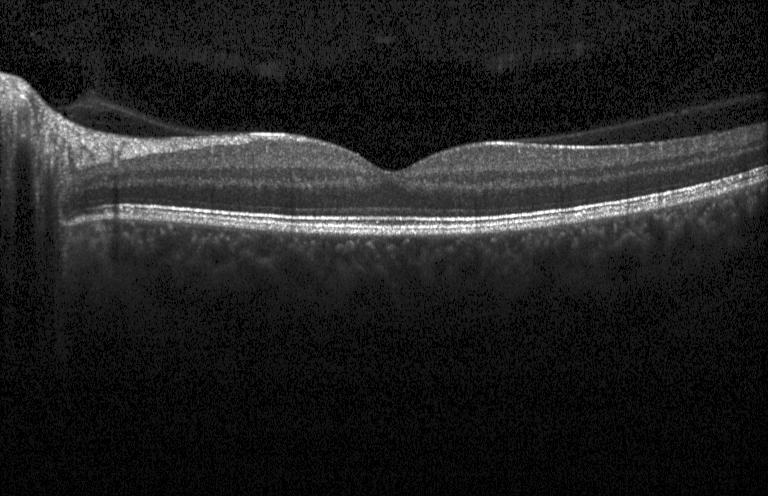
Heidelberg Spectralis; retinal OCT cross-section; macular scan
This B-scan demonstrates no choroidal neovascularization, diabetic macular edema, or drusen.